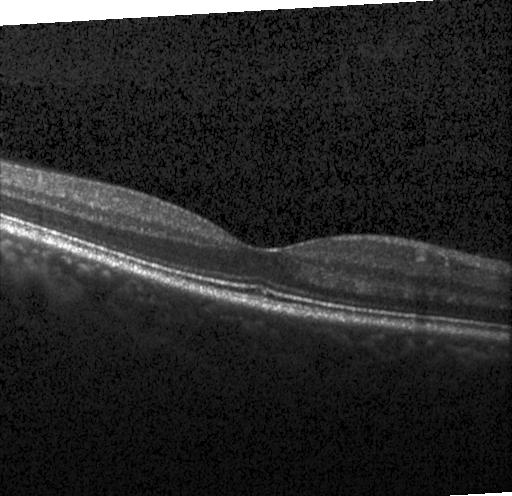
SD-OCT. Macular scan. Instrument: Heidelberg Spectralis. Retinal OCT cross-section
No choroidal neovascularization, diabetic macular edema, or drusen.